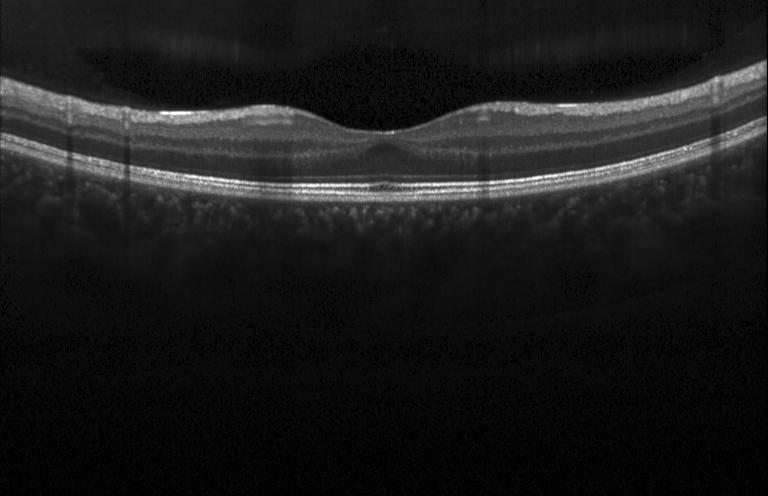 Assessment: no evidence of CNV, DME, or drusen.